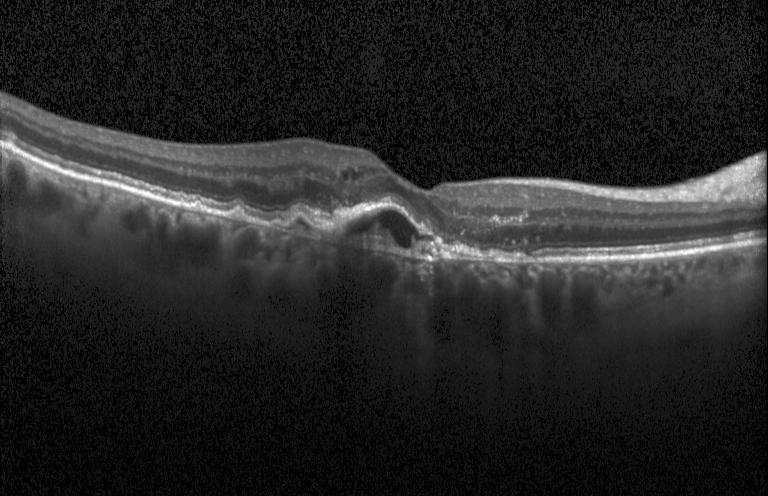

Retinal OCT cross-section showing choroidal neovascularization (CNV).